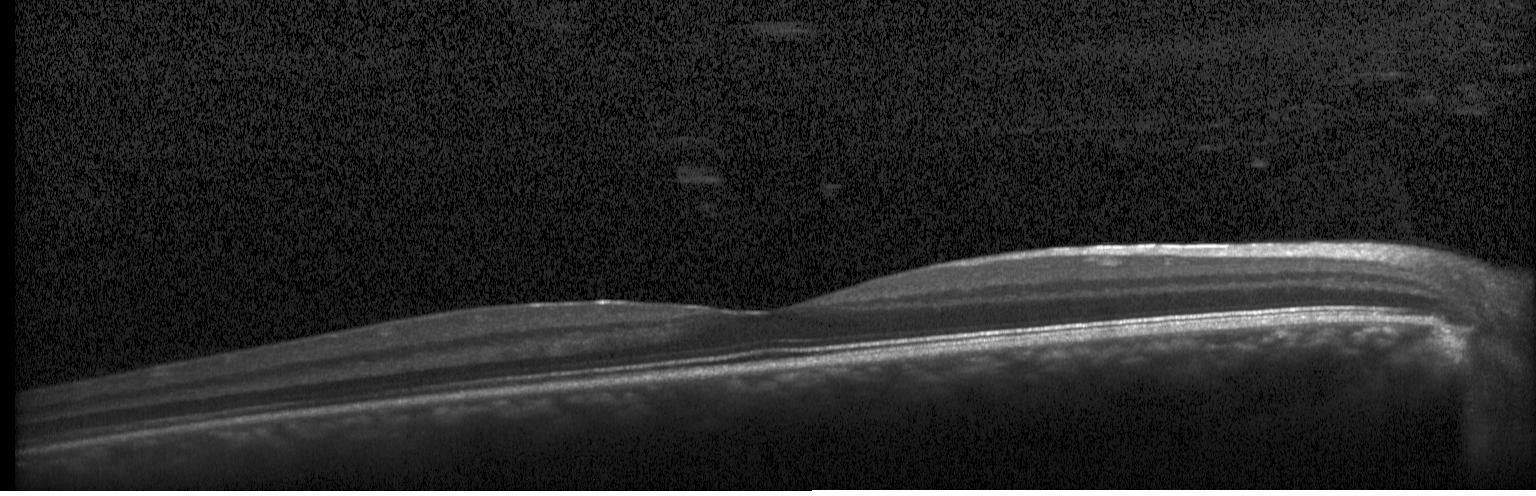
Macular OCT demonstrating no evidence of choroidal neovascularization, diabetic macular edema, or drusen.